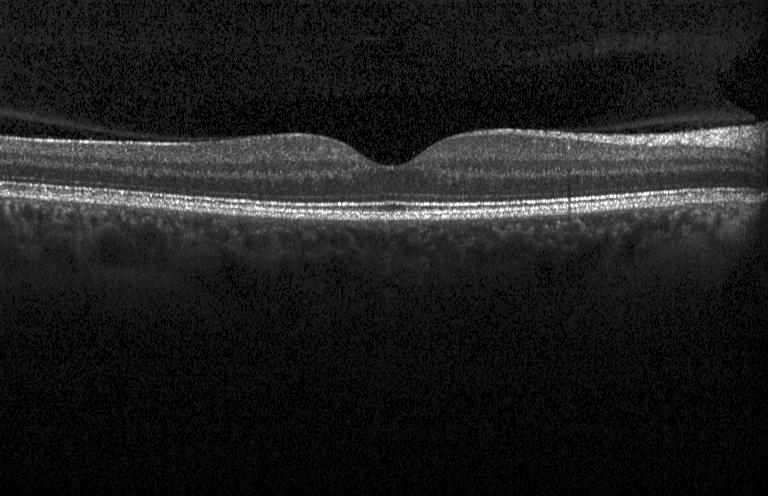 OCT B-scan showing neither choroidal neovascularization, diabetic macular edema, nor drusen.